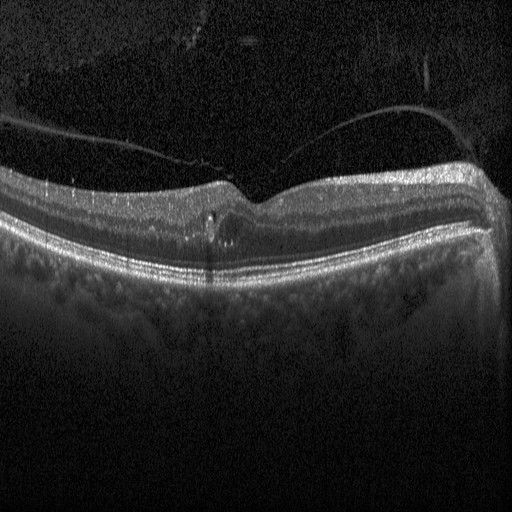
Dx: diabetic macular edema (DME).